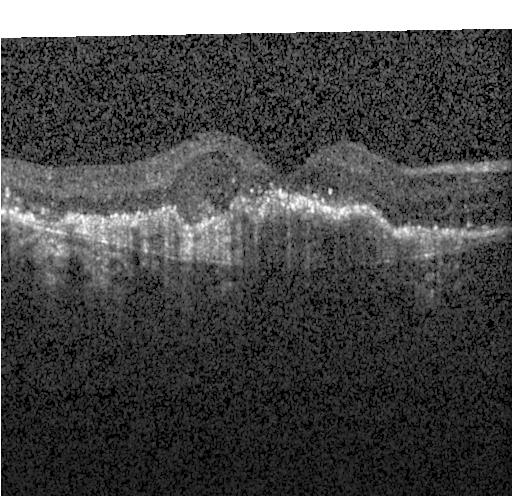
Optical coherence tomography B-scan, macular scan.
Diagnosis: a choroidal neovascular membrane.